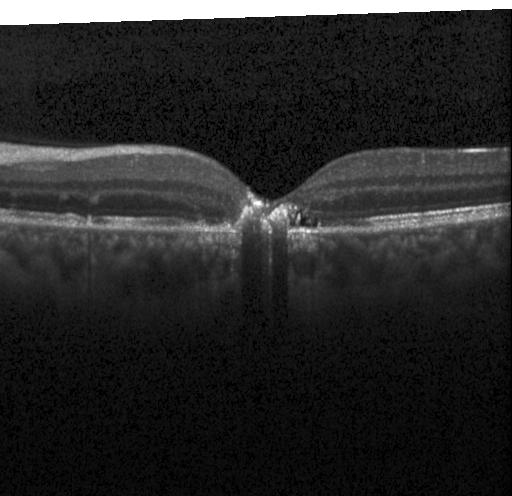

Heidelberg Spectralis. Optical coherence tomography B-scan. Impression: choroidal neovascularization (CNV).